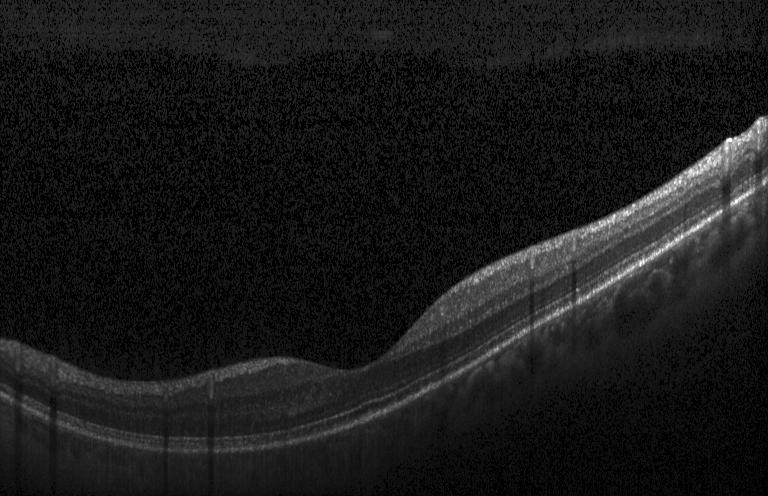
Retinal OCT B-scan. Impression: no CNV, no DME, and no drusen.